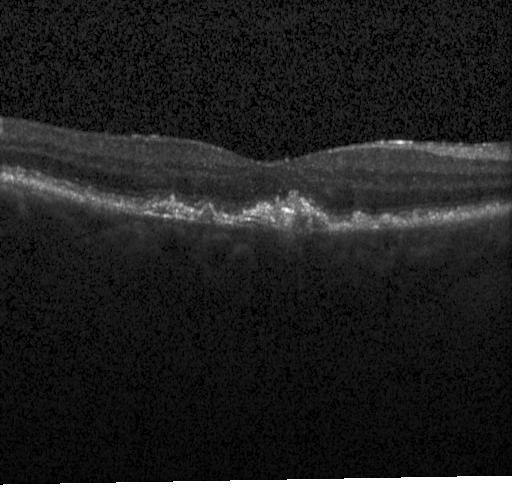
OCT B-scan. Finding: choroidal neovascularization (CNV).